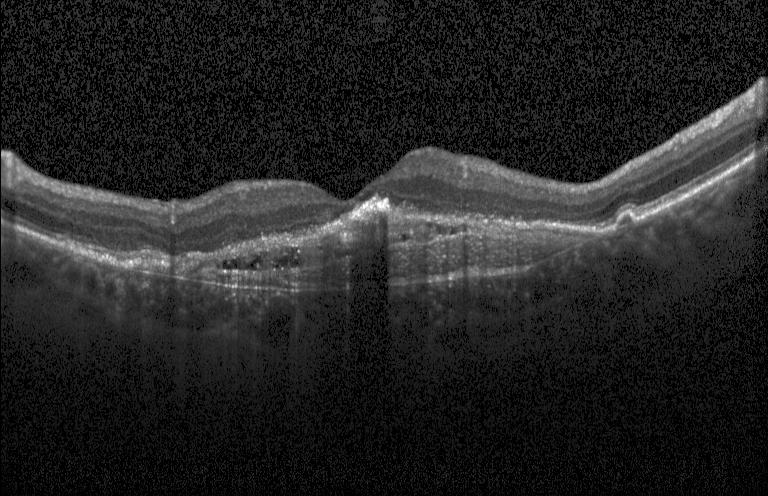
OCT B-scan. Diagnosis: choroidal neovascularization.